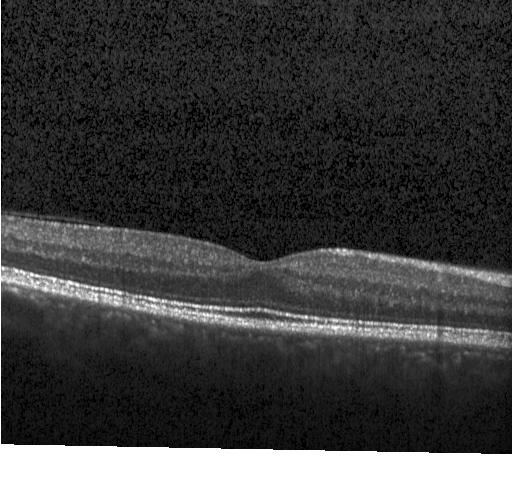
Assessment: no choroidal neovascularization, no diabetic macular edema, and no drusen.